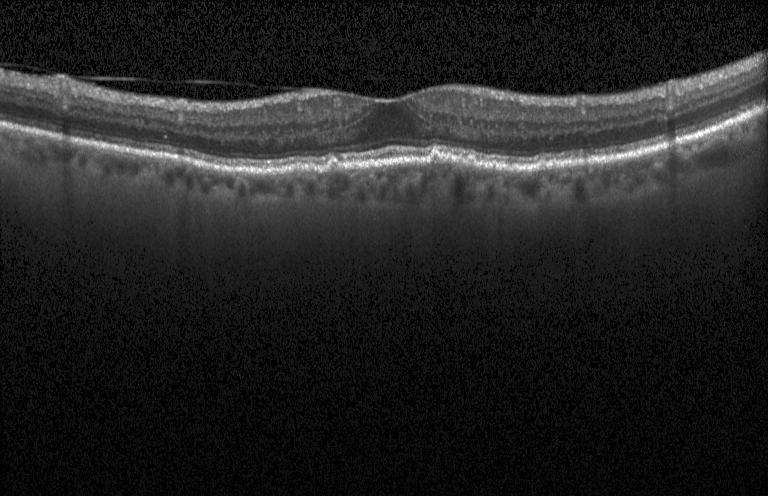 Retinal OCT cross-section showing sub-RPE drusenoid deposits.